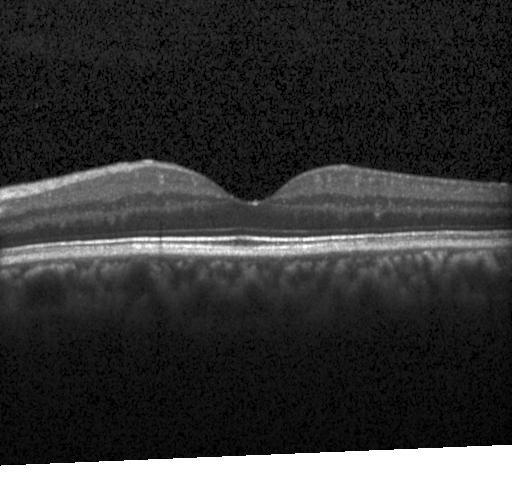

Macular OCT demonstrating neither CNV, DME, nor drusen.